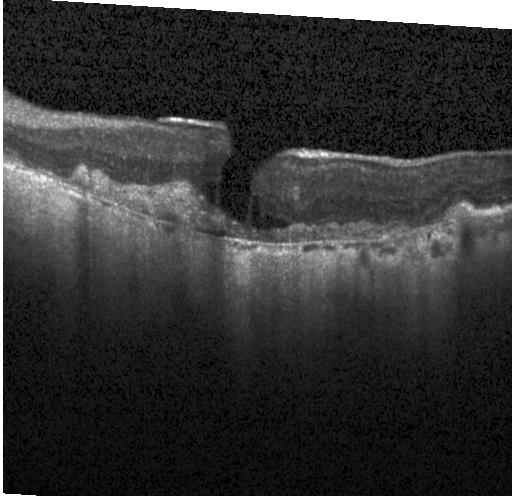 Impression: choroidal neovascularization.